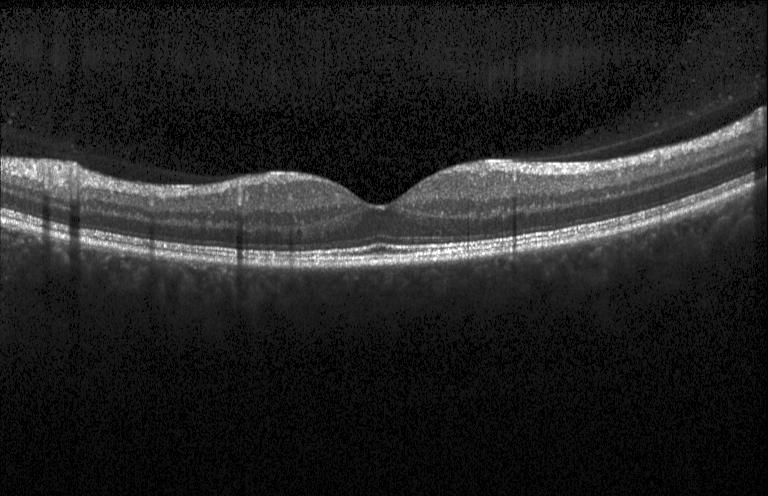 Spectral-domain optical coherence tomography · optical coherence tomography B-scan.
This B-scan demonstrates neither choroidal neovascularization, diabetic macular edema, nor drusen.